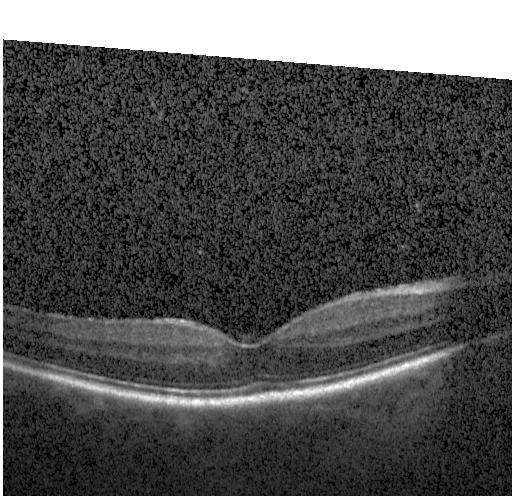
Heidelberg Spectralis, macular scan, optical coherence tomography scan
Assessment: no CNV, DME, or drusen.